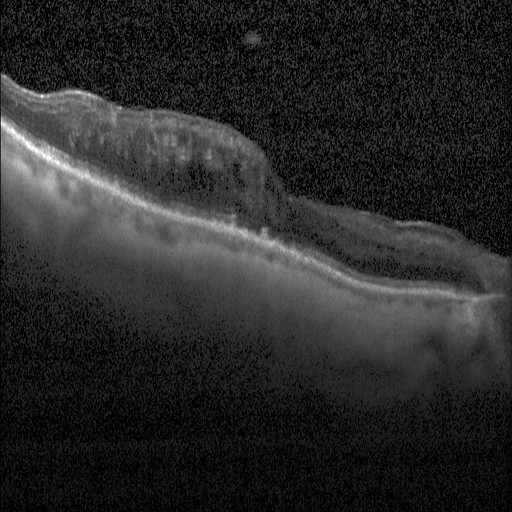

Macular OCT: diabetic macular edema (DME).